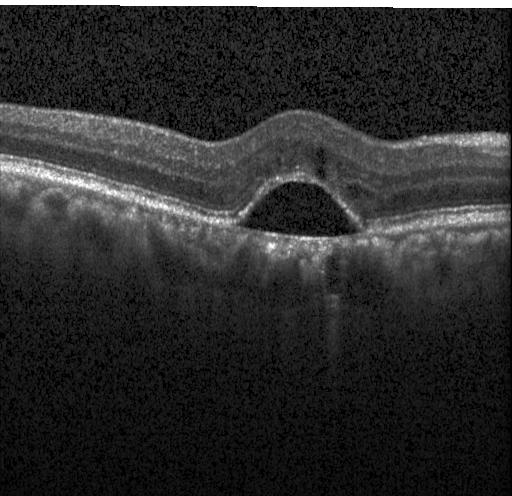
Horizontal scan through the fovea · Heidelberg Spectralis · optical coherence tomography scan — Diagnosis: a choroidal neovascular membrane.